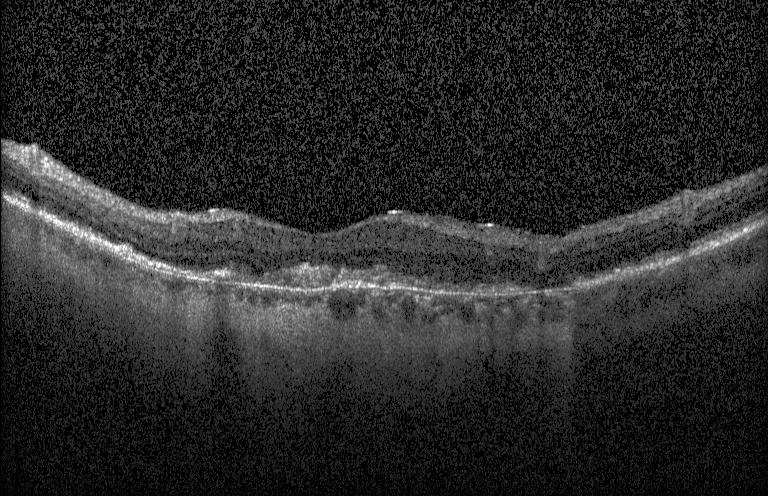
The scan shows choroidal neovascularization (CNV).